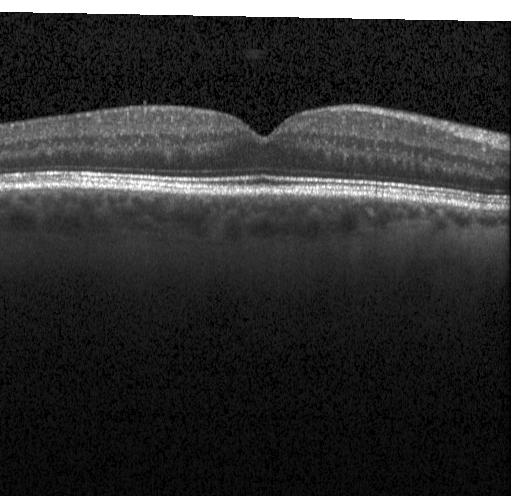
OCT line scan.
OCT finding: no CNV, DME, or drusen.